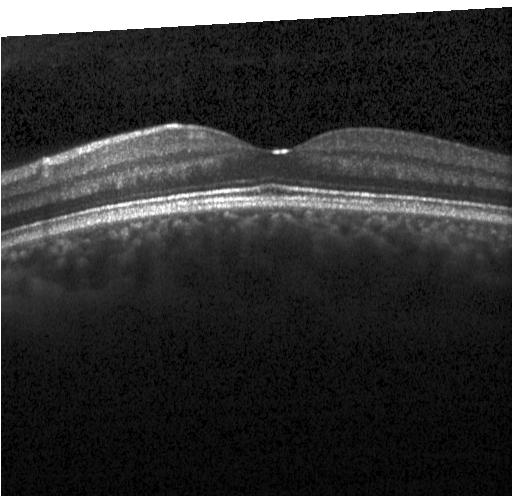
Heidelberg Spectralis OCT system; horizontal scan through the fovea; spectral-domain optical coherence tomography; OCT line scan. The scan shows no evidence of CNV, DME, or drusen.